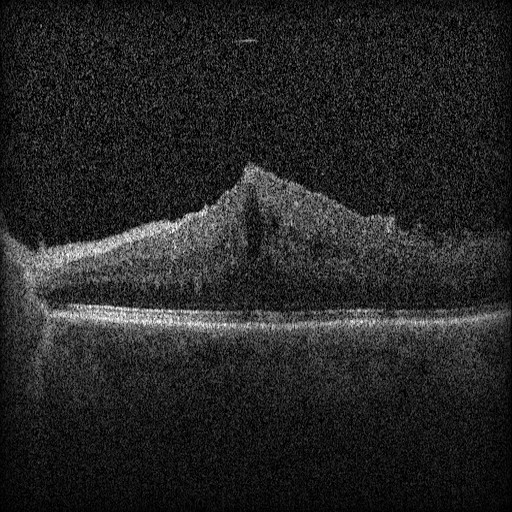
Retinal OCT B-scan. This B-scan demonstrates DME.